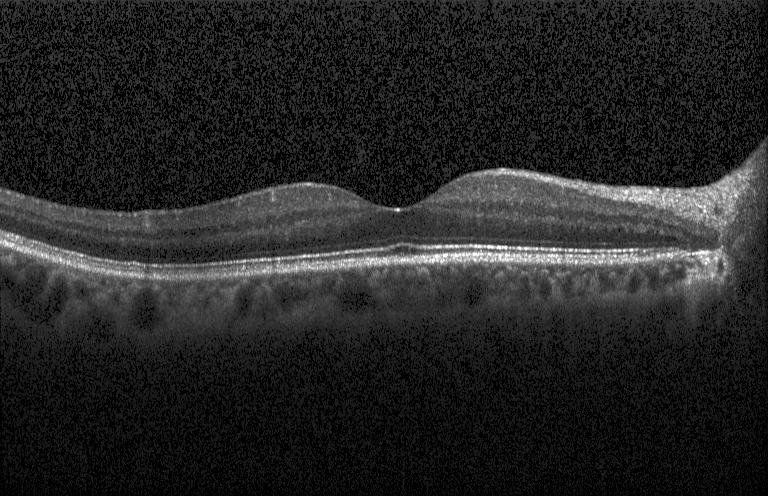 Dx: neither CNV, DME, nor drusen.